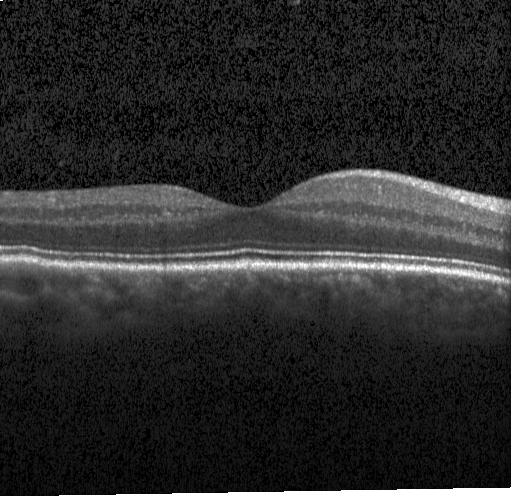

OCT line scan, instrument: Heidelberg Spectralis, SD-OCT
Diagnosis: no choroidal neovascularization, diabetic macular edema, or drusen.